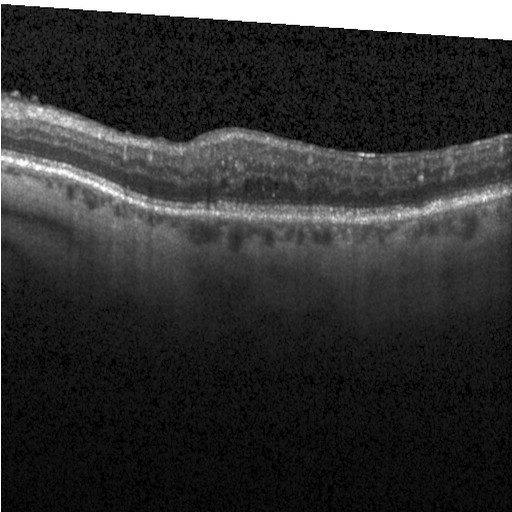 OCT B-scan. Macular scan.
Diagnosis: DME.